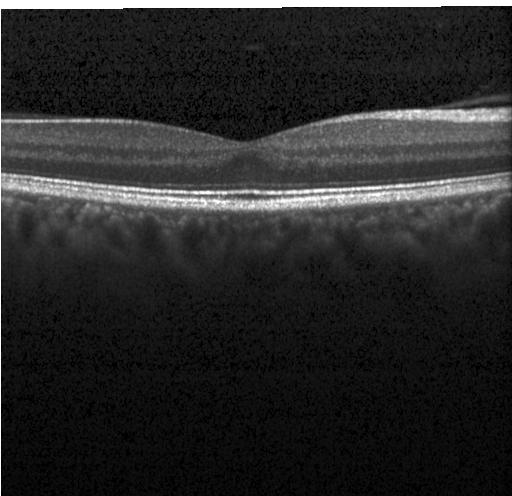 Spectral-domain optical coherence tomography, retinal OCT cross-section — Finding: no CNV, no DME, and no drusen.